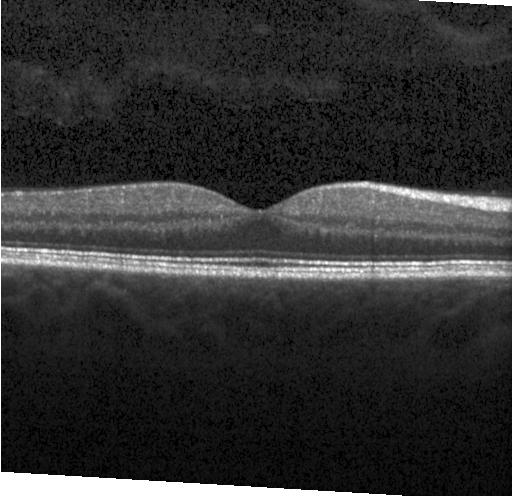

Heidelberg Spectralis OCT system; spectral-domain optical coherence tomography; macular scan; OCT B-scan.
Impression: no CNV, no DME, and no drusen.